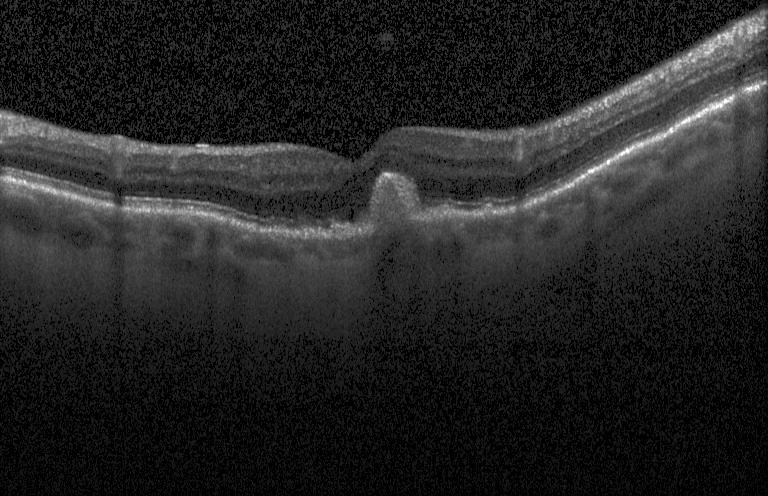

Impression: sub-RPE drusenoid deposits.